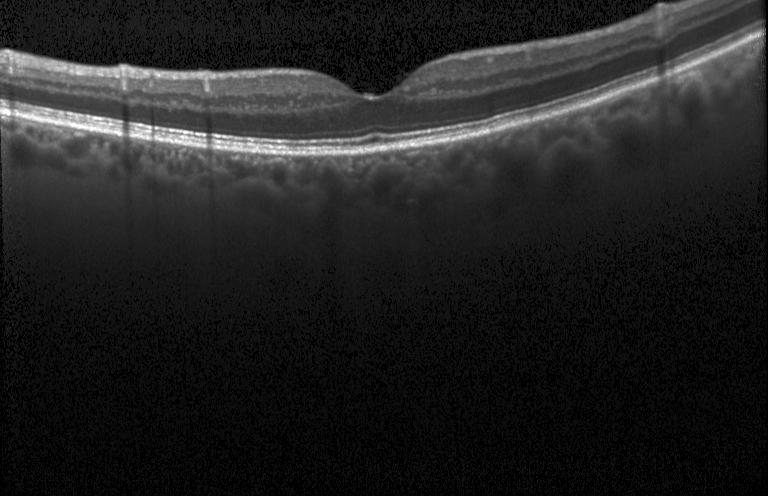
Optical coherence tomography scan
No choroidal neovascularization, no diabetic macular edema, and no drusen.